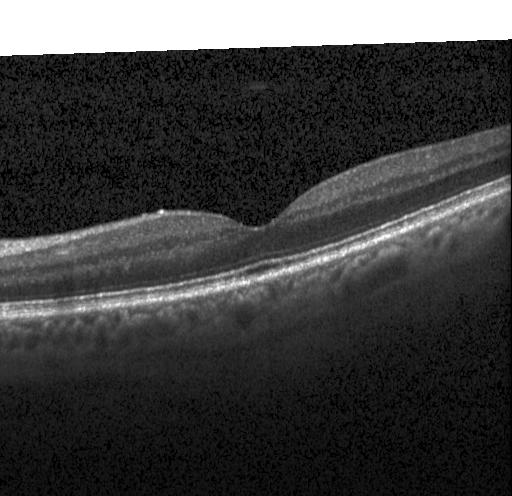 Fovea-centered; Heidelberg Spectralis OCT system; retinal OCT B-scan. Assessment: no choroidal neovascularization, no diabetic macular edema, and no drusen.